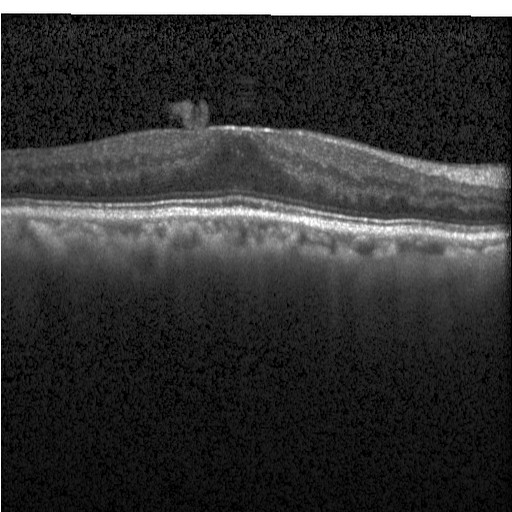 Spectral-domain OCT, optical coherence tomography B-scan, horizontal scan through the fovea.
Diabetic macular edema.